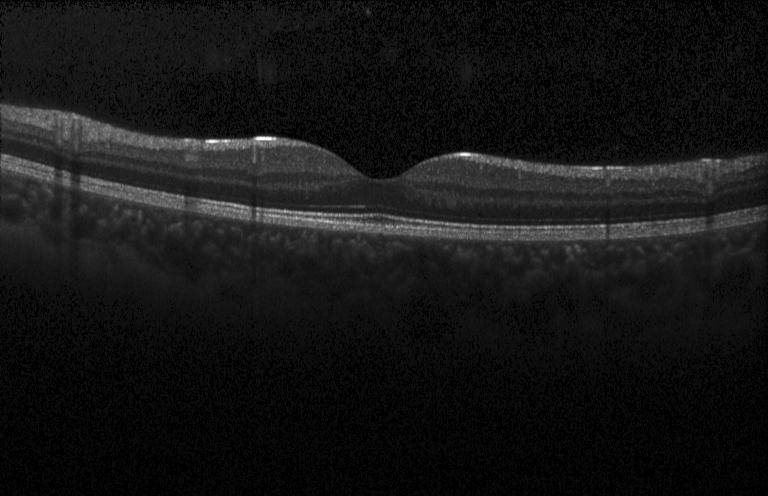
Spectral-domain OCT · retinal OCT cross-section
Macular OCT: no choroidal neovascularization, no diabetic macular edema, and no drusen.